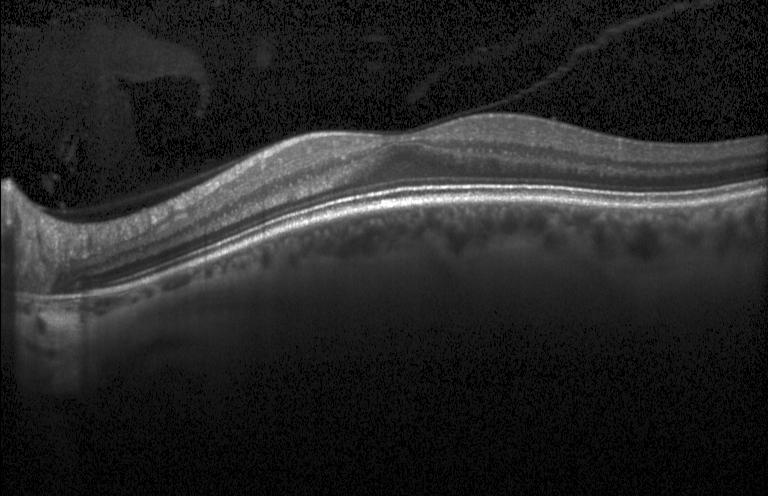

This B-scan demonstrates neither choroidal neovascularization, diabetic macular edema, nor drusen.